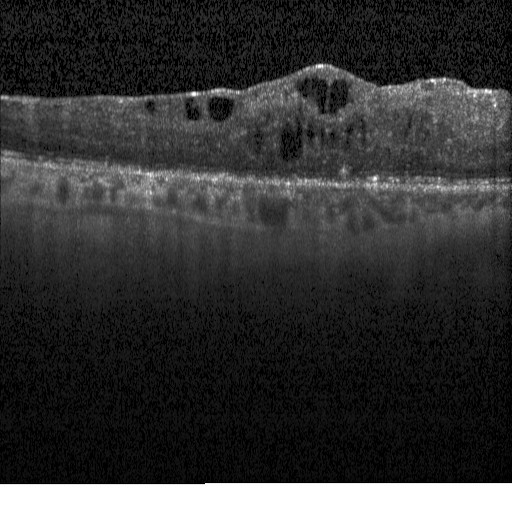
Spectral-domain optical coherence tomography, OCT B-scan
Diabetic macular edema (DME).